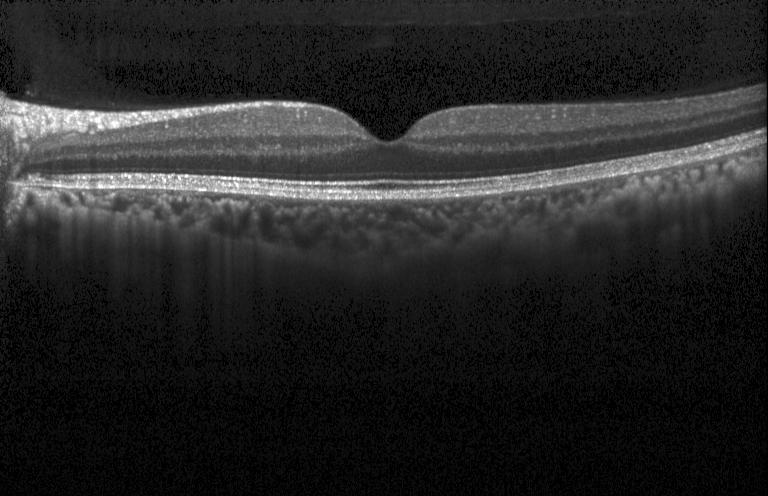 Heidelberg Spectralis OCT system; spectral-domain OCT; optical coherence tomography B-scan; centered on the fovea.
Dx: no choroidal neovascularization, no diabetic macular edema, and no drusen.